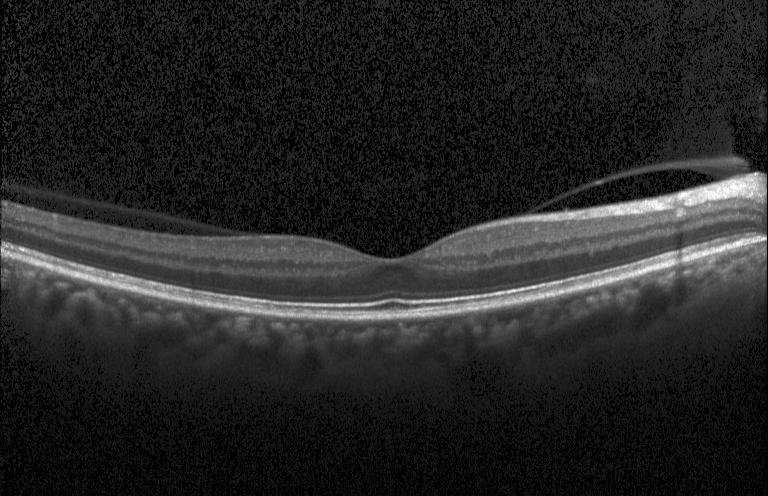
OCT line scan; Heidelberg Spectralis. The scan shows neither CNV, DME, nor drusen.